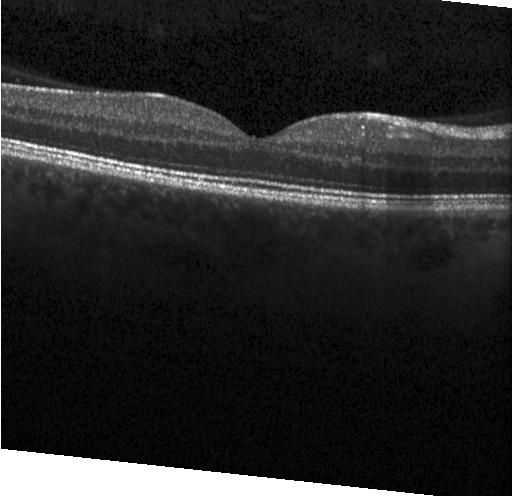

Assessment: no choroidal neovascularization, no diabetic macular edema, and no drusen.